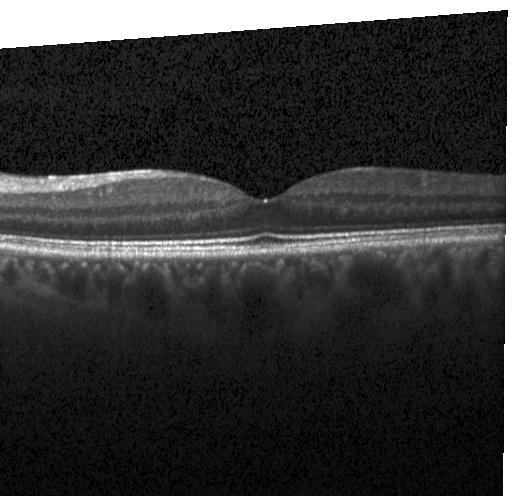
Macular scan · retinal OCT cross-section. Impression: neither choroidal neovascularization, diabetic macular edema, nor drusen.